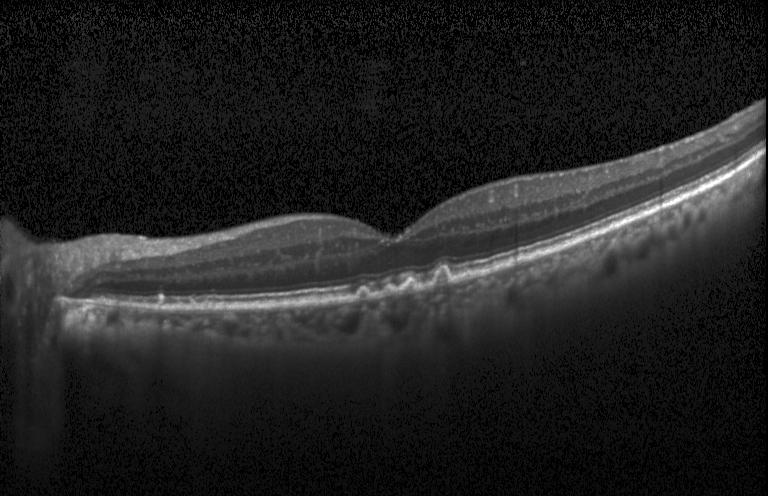
Centered on the fovea. OCT line scan.
Diagnosis: drusen.